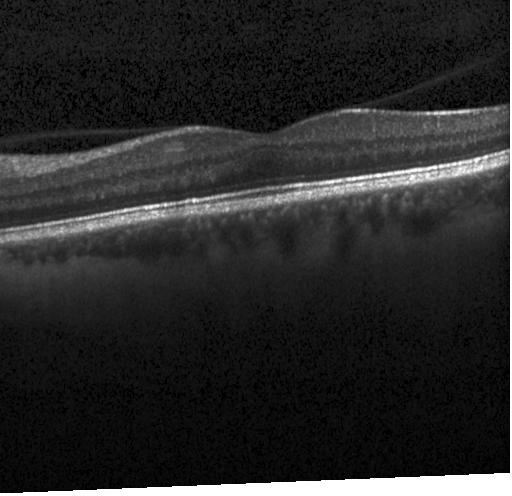

Retinal OCT cross-section; instrument: Heidelberg Spectralis.
Finding: no evidence of choroidal neovascularization, diabetic macular edema, or drusen.